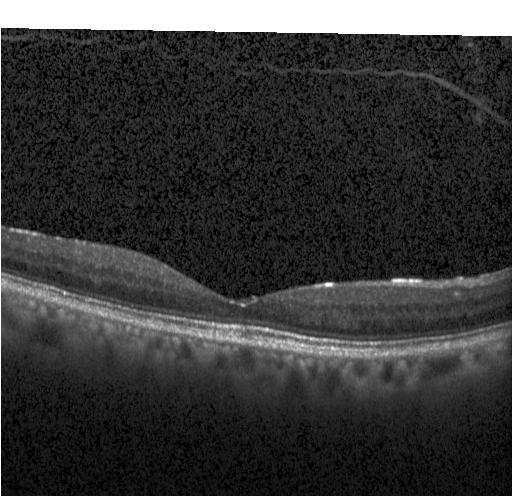

Macular scan, retinal OCT B-scan, spectral-domain OCT
Diagnosis: no choroidal neovascularization, no diabetic macular edema, and no drusen.